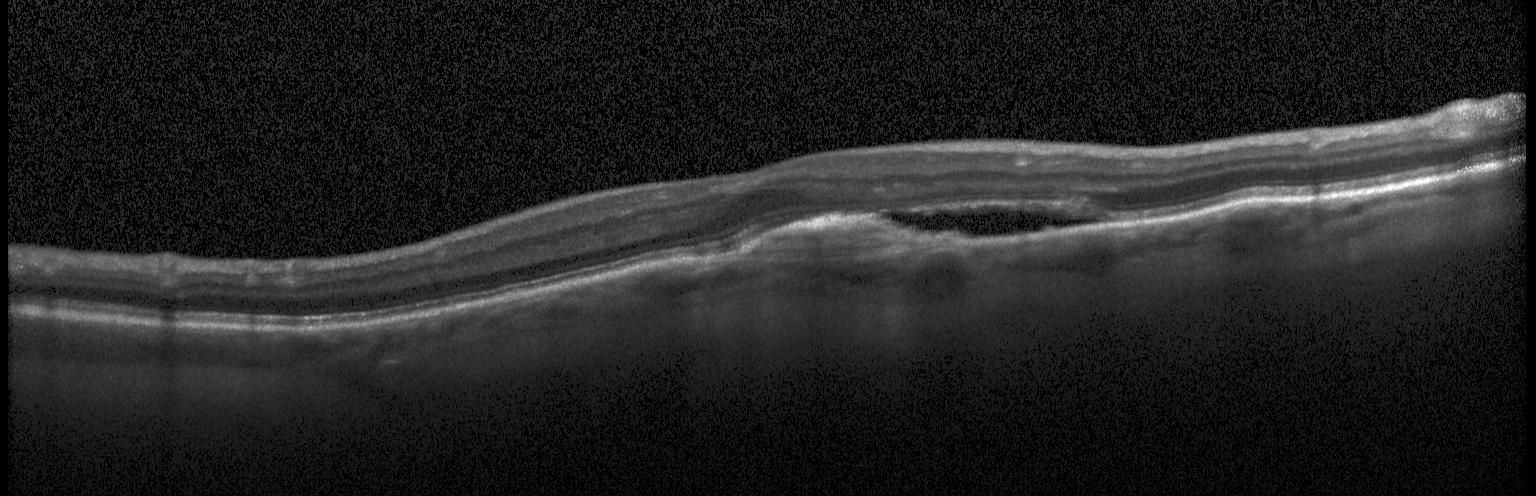
Macular OCT: choroidal neovascularization (CNV).